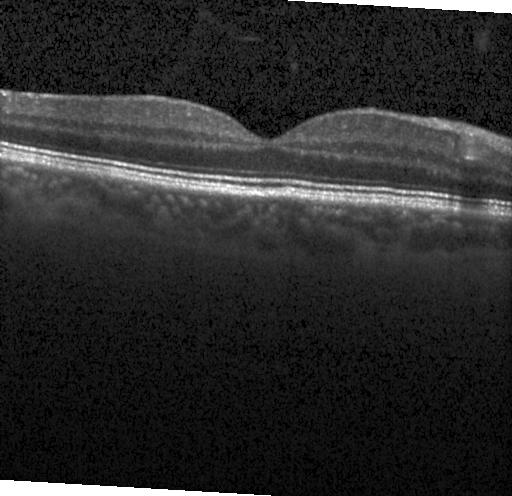
Finding: no evidence of choroidal neovascularization, diabetic macular edema, or drusen.